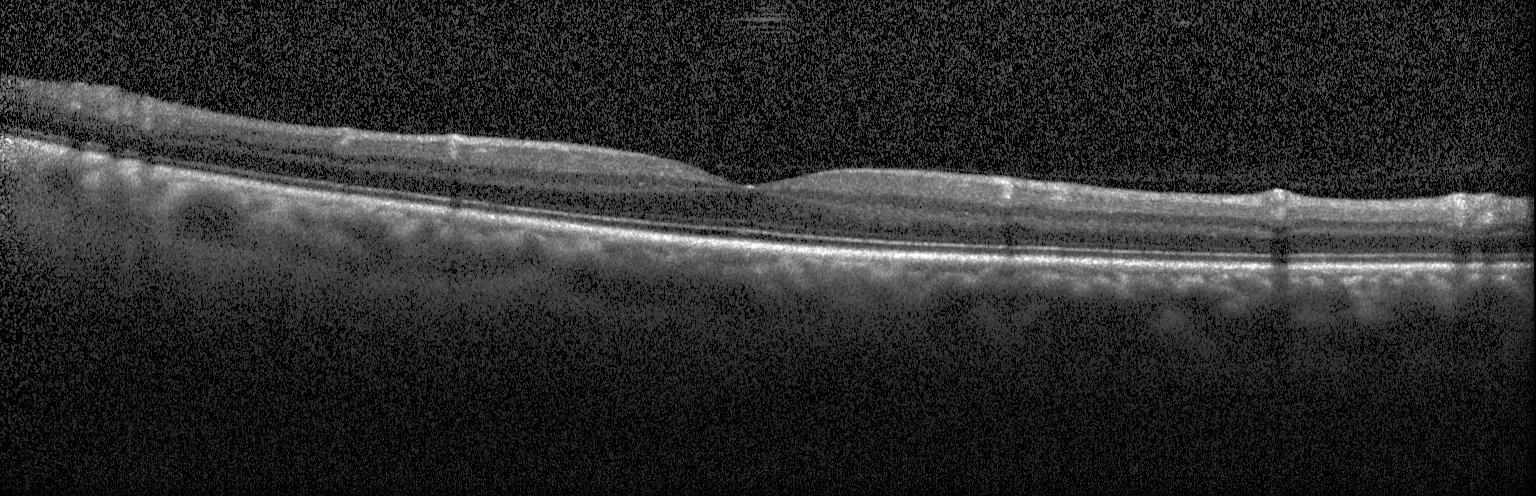

Dx: no choroidal neovascularization, diabetic macular edema, or drusen.